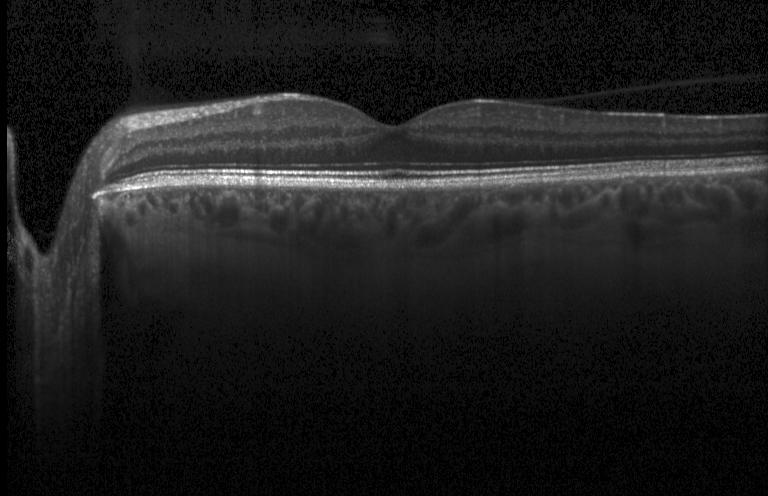

Optical coherence tomography B-scan. Heidelberg Spectralis OCT system.
Assessment: no evidence of choroidal neovascularization, diabetic macular edema, or drusen.